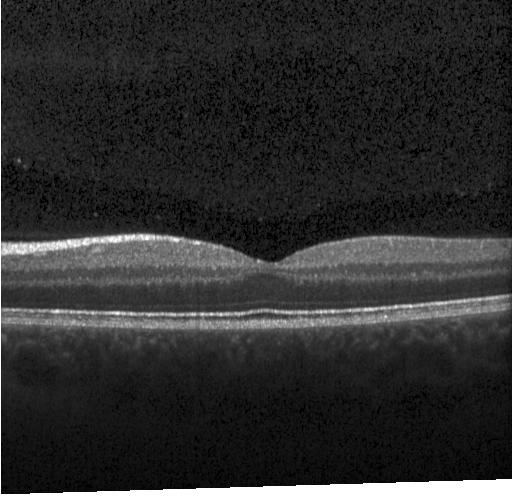

Fovea-centered, retinal OCT B-scan, Heidelberg Spectralis, spectral-domain OCT — Finding: no choroidal neovascularization, diabetic macular edema, or drusen.